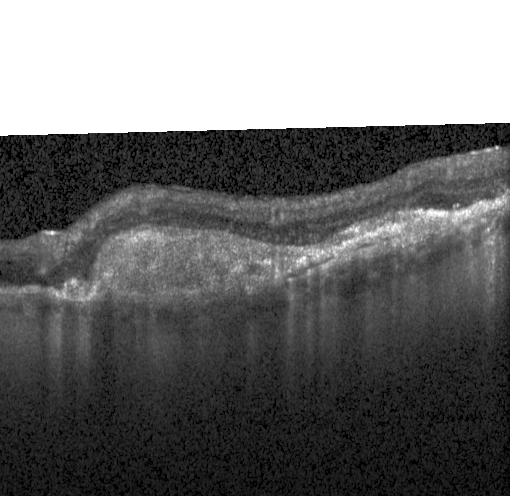

Fovea-centered; instrument: Heidelberg Spectralis; optical coherence tomography B-scan.
Impression: a choroidal neovascular membrane.